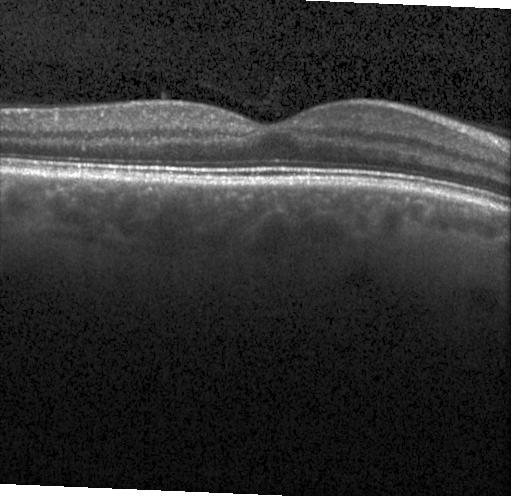 Through the macula; spectral-domain OCT; Heidelberg Spectralis; retinal OCT B-scan.
The scan shows no choroidal neovascularization, diabetic macular edema, or drusen.